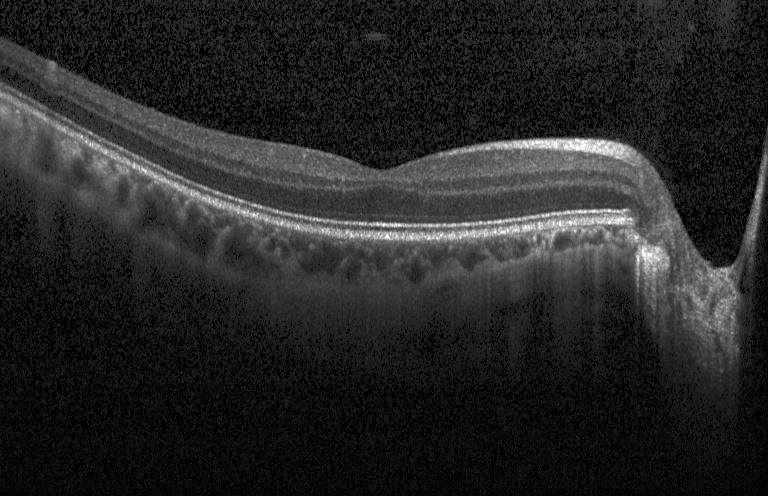 Fovea-centered · optical coherence tomography scan · SD-OCT · acquired on a Heidelberg Spectralis. Impression: no choroidal neovascularization, no diabetic macular edema, and no drusen.